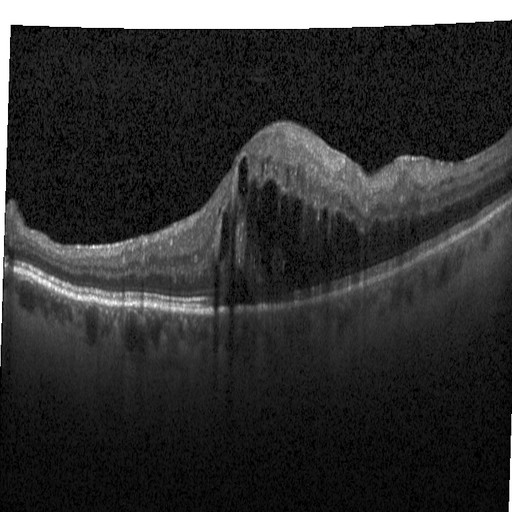

Retinal OCT cross-section showing DME.